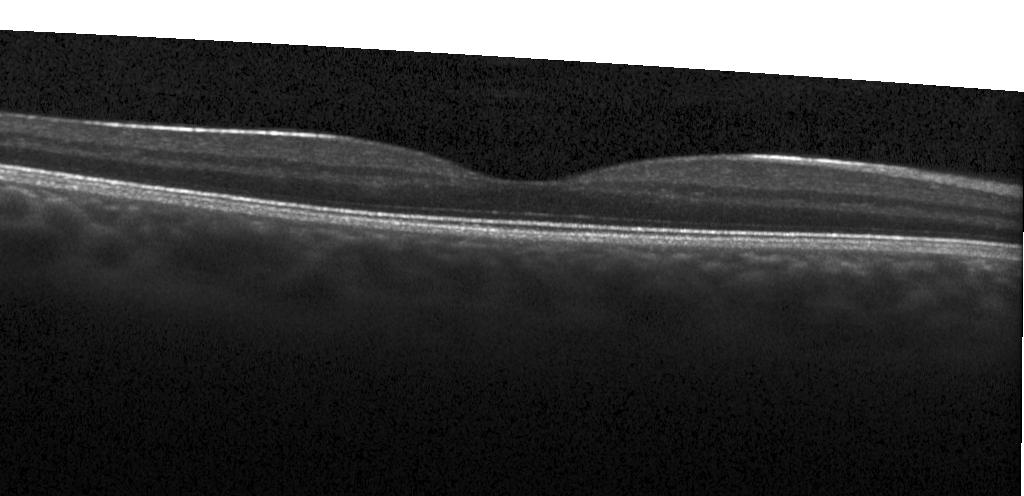
Macular OCT: no choroidal neovascularization, diabetic macular edema, or drusen.